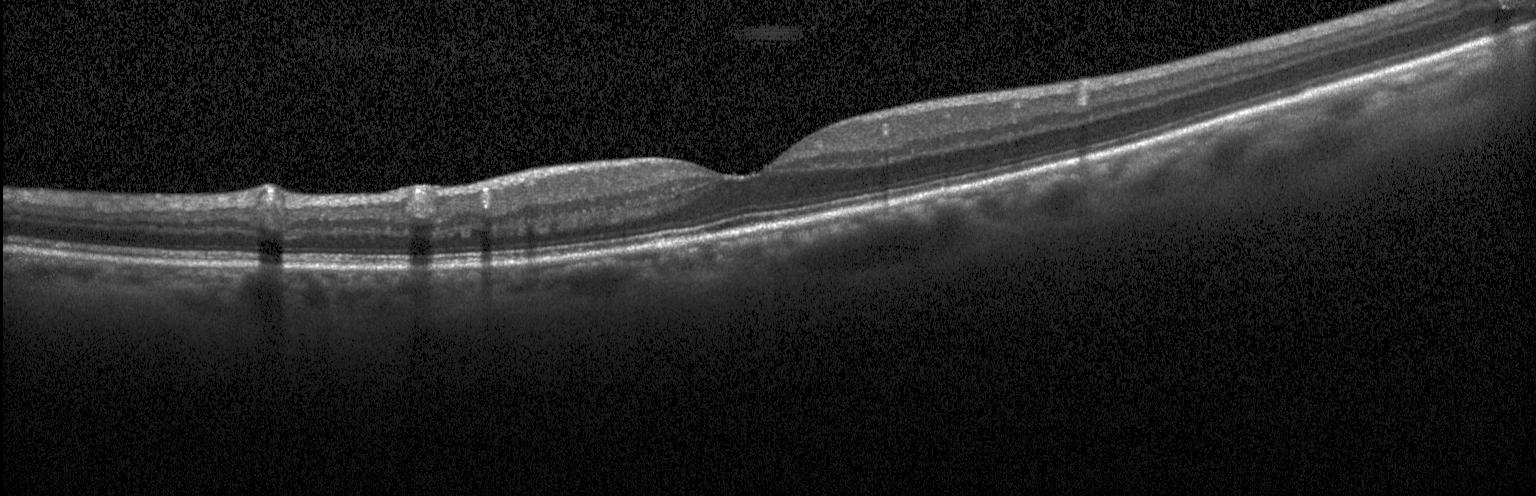 Diagnosis: neither choroidal neovascularization, diabetic macular edema, nor drusen.